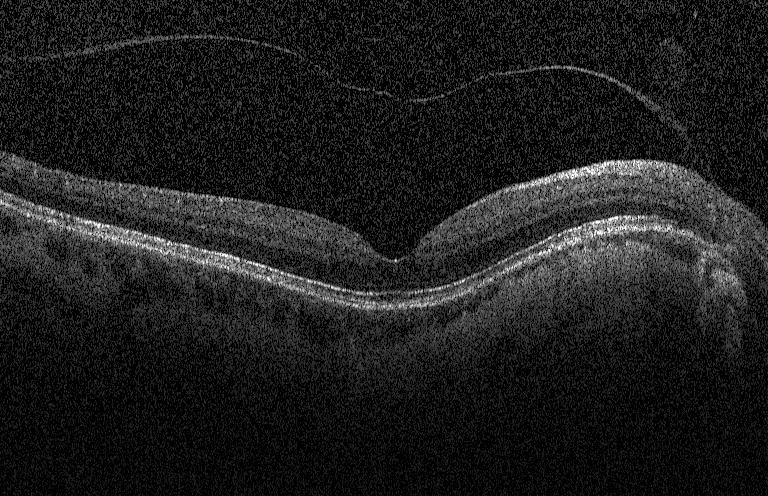 OCT line scan; spectral-domain OCT; centered on the fovea; instrument: Heidelberg Spectralis.
No evidence of choroidal neovascularization, diabetic macular edema, or drusen.